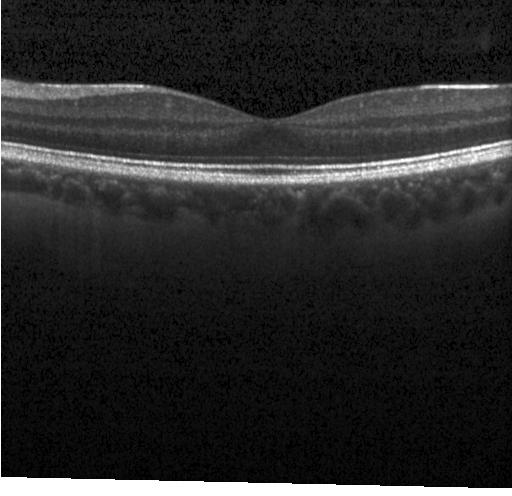
This B-scan demonstrates no choroidal neovascularization, diabetic macular edema, or drusen.